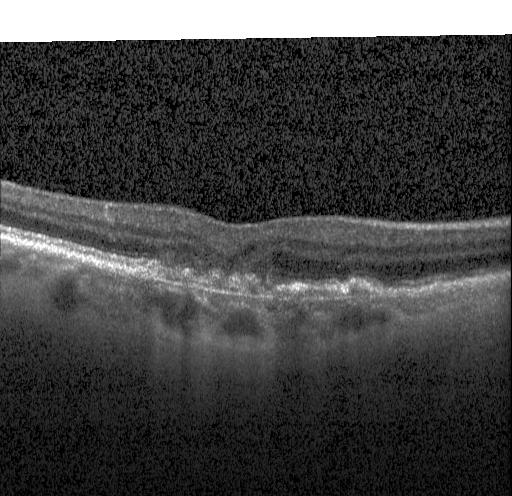

Spectral-domain OCT B-scan: choroidal neovascularization (CNV).